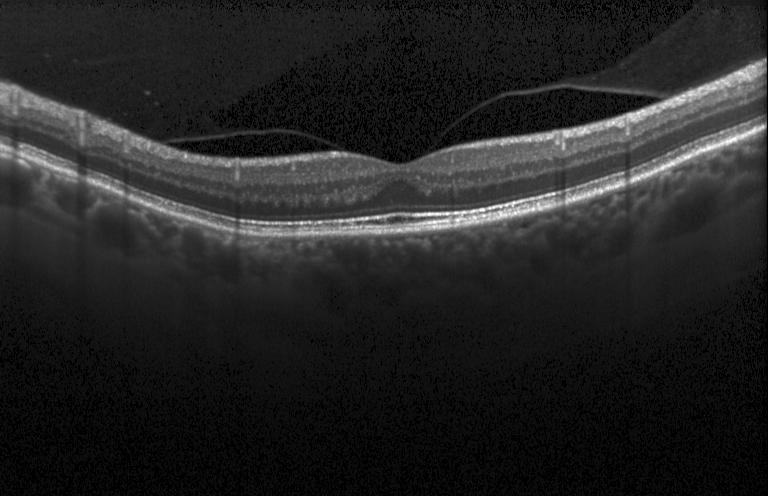

Optical coherence tomography scan. Impression: neither choroidal neovascularization, diabetic macular edema, nor drusen.